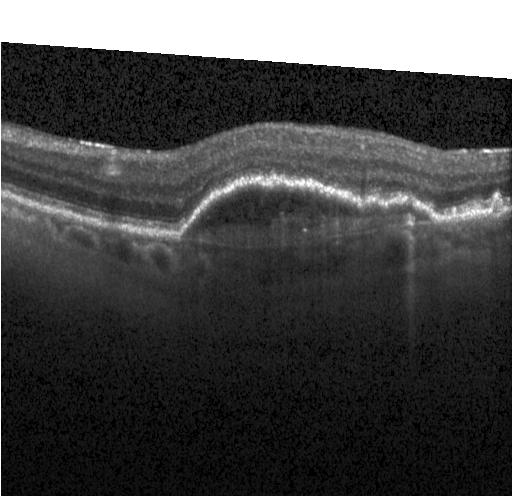

Diagnosis: choroidal neovascularization (CNV).